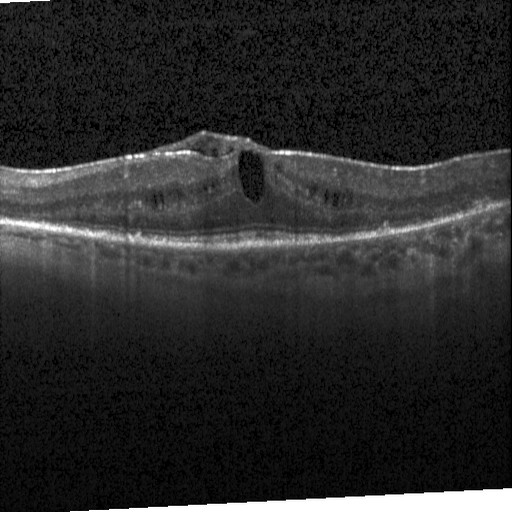 Retinal OCT B-scan — Dx: DME.